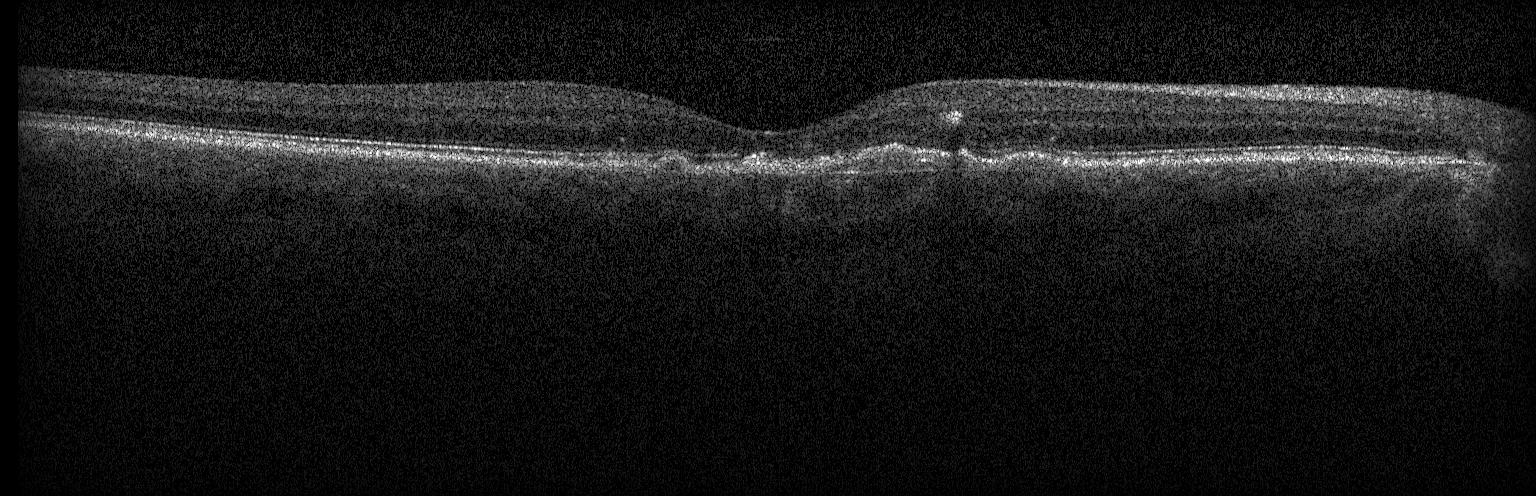

Diagnosis: a choroidal neovascular membrane.